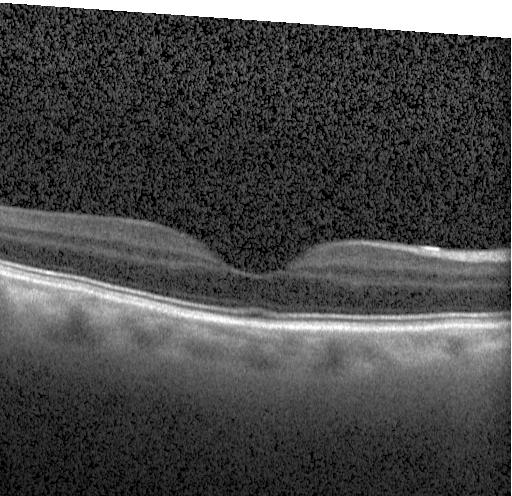 Dx: no evidence of CNV, DME, or drusen.